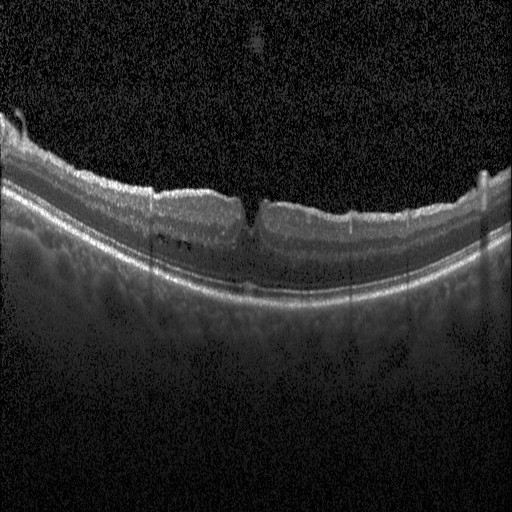

Optical coherence tomography B-scan. Horizontal scan through the fovea.
OCT finding: diabetic macular edema (DME).